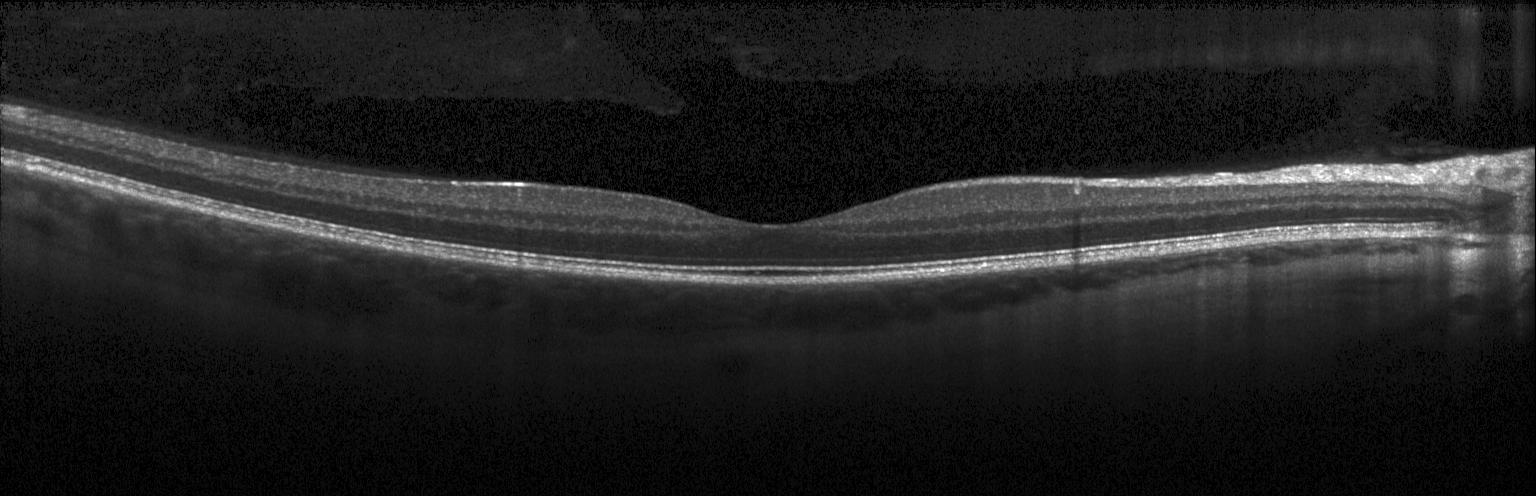

Optical coherence tomography scan, instrument: Heidelberg Spectralis.
Diagnosis: no choroidal neovascularization, diabetic macular edema, or drusen.